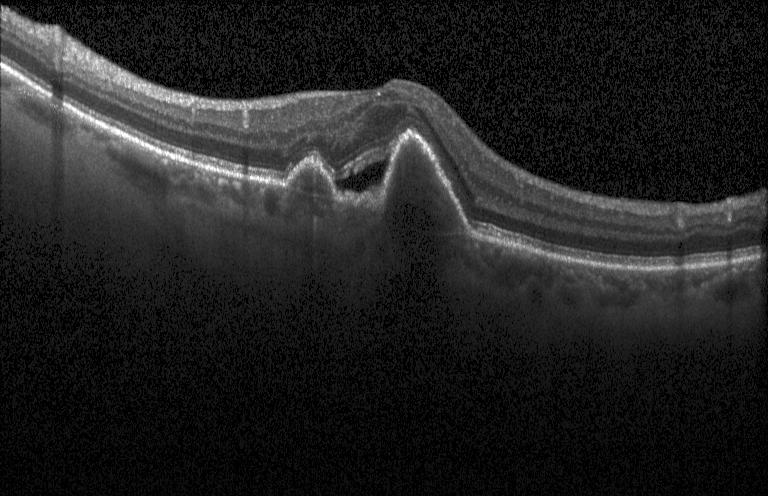
Spectral-domain OCT, horizontal scan through the fovea, acquired on a Heidelberg Spectralis, retinal OCT cross-section.
The scan shows a choroidal neovascular membrane.